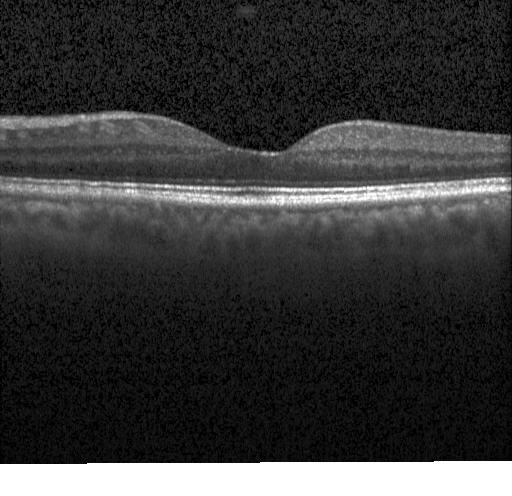
The scan shows no choroidal neovascularization, no diabetic macular edema, and no drusen.